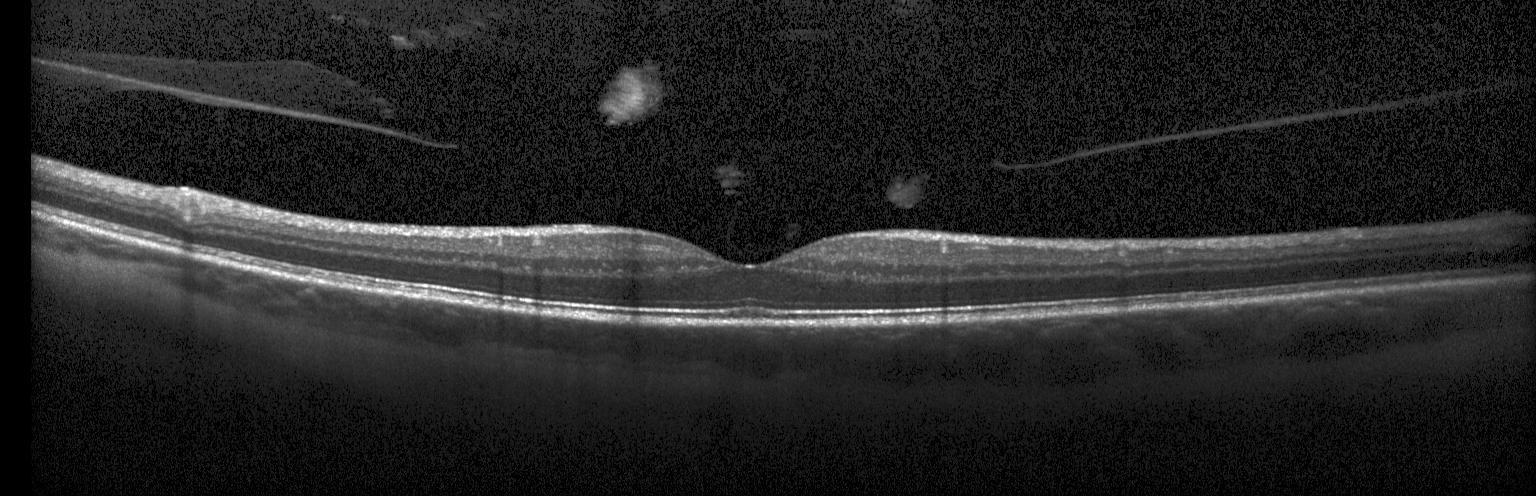

Retinal OCT B-scan.
Finding: neither CNV, DME, nor drusen.